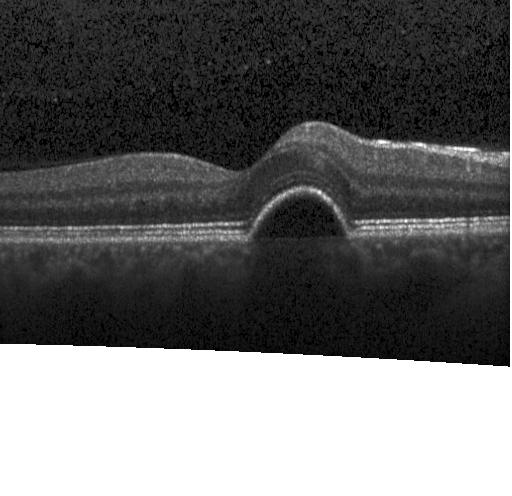

Horizontal scan through the fovea. Retinal OCT B-scan. Spectral-domain optical coherence tomography. Heidelberg Spectralis
The scan shows a choroidal neovascular membrane.